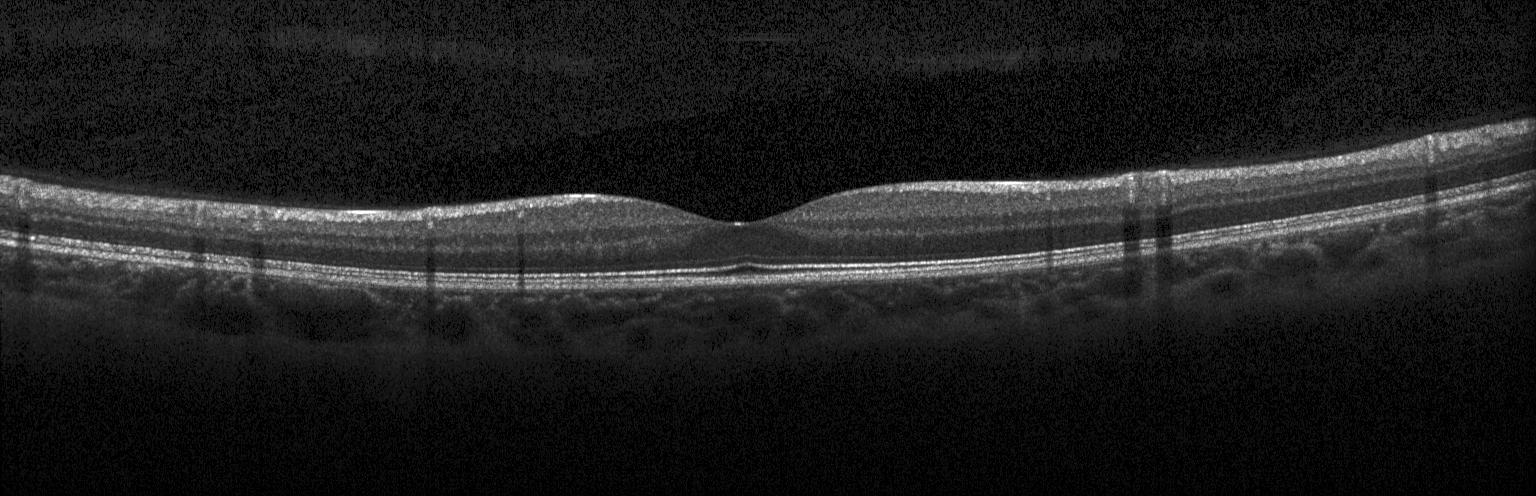 Fovea-centered, optical coherence tomography B-scan.
Impression: no choroidal neovascularization, diabetic macular edema, or drusen.